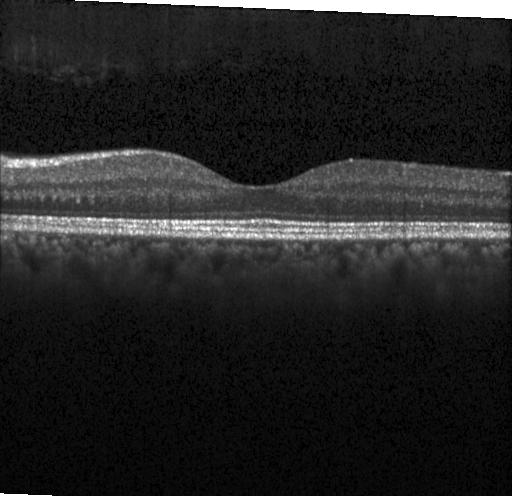
Diagnosis: neither CNV, DME, nor drusen.